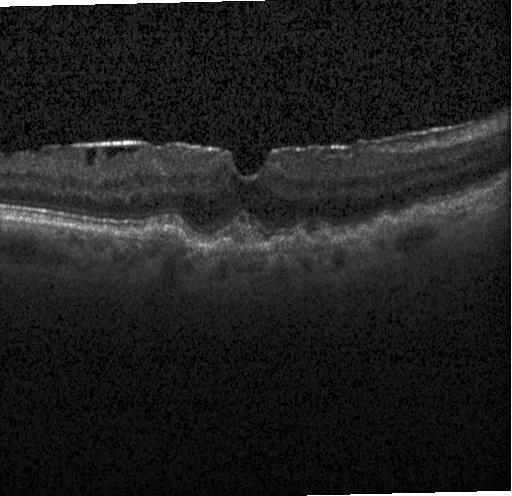 OCT B-scan showing drusen.